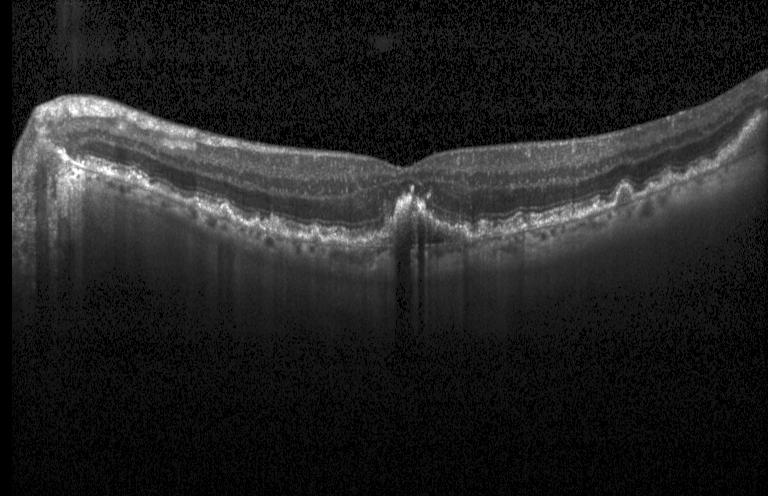

Acquired on a Heidelberg Spectralis, OCT line scan — A choroidal neovascular membrane.